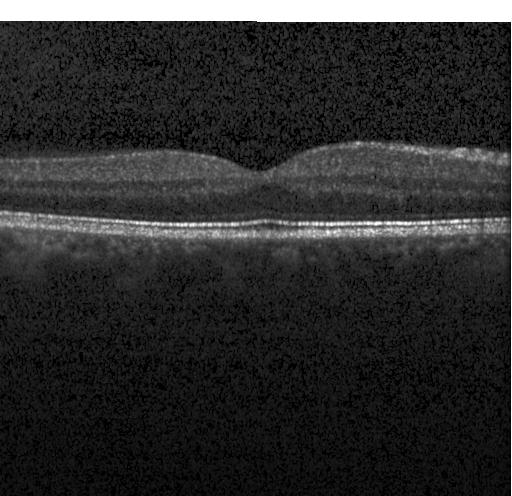 This B-scan demonstrates no CNV, no DME, and no drusen.